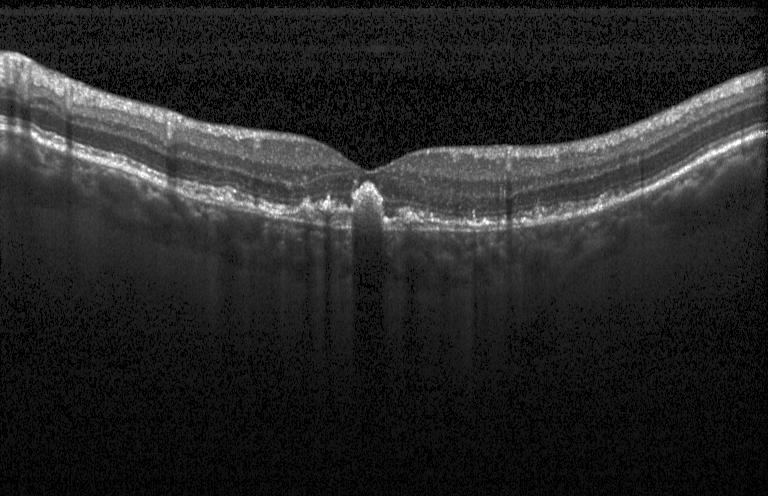

Retinal OCT B-scan. The scan shows a choroidal neovascular membrane.